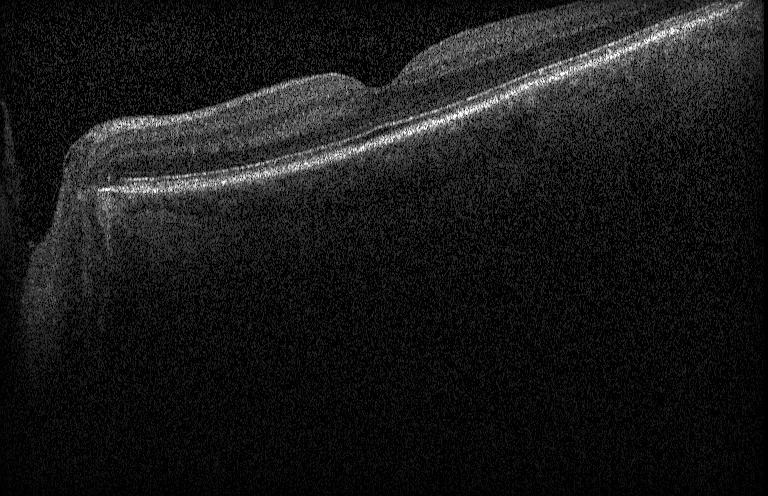
This B-scan demonstrates neither choroidal neovascularization, diabetic macular edema, nor drusen.